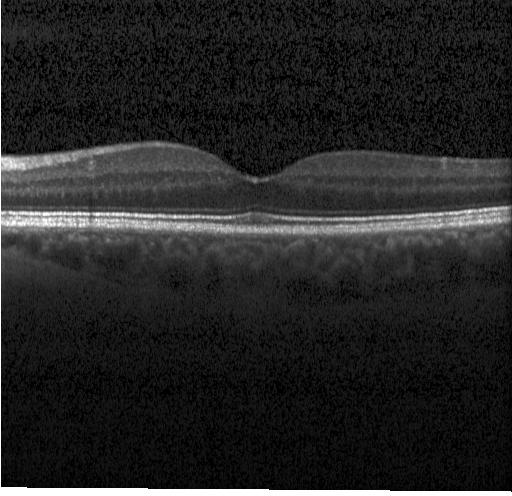 OCT line scan · Heidelberg Spectralis. Assessment: no choroidal neovascularization, diabetic macular edema, or drusen.